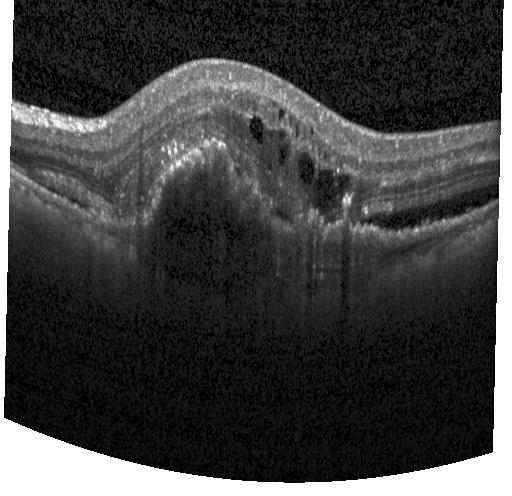
Retinal OCT B-scan. Diagnosis: choroidal neovascularization (CNV).